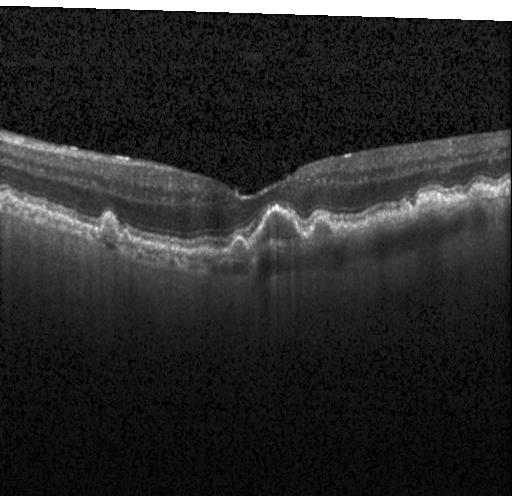
Finding: sub-RPE drusenoid deposits.